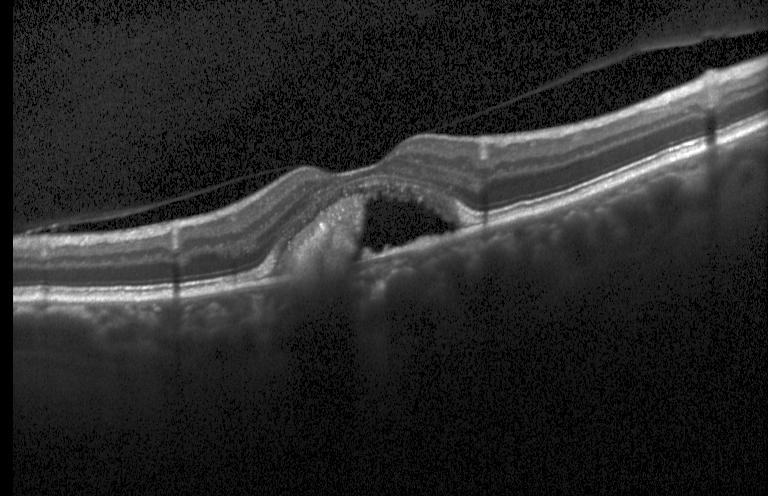 The scan shows a choroidal neovascular membrane.